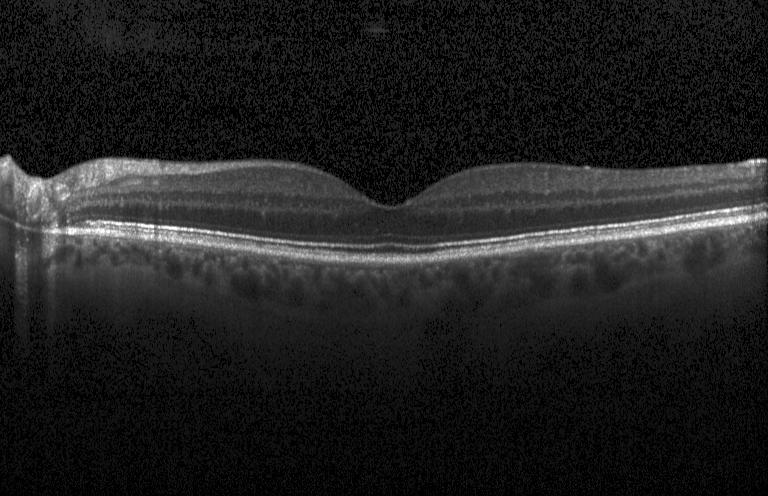

Retinal OCT cross-section · Heidelberg Spectralis · spectral-domain OCT · macular scan. Macular OCT: neither choroidal neovascularization, diabetic macular edema, nor drusen.